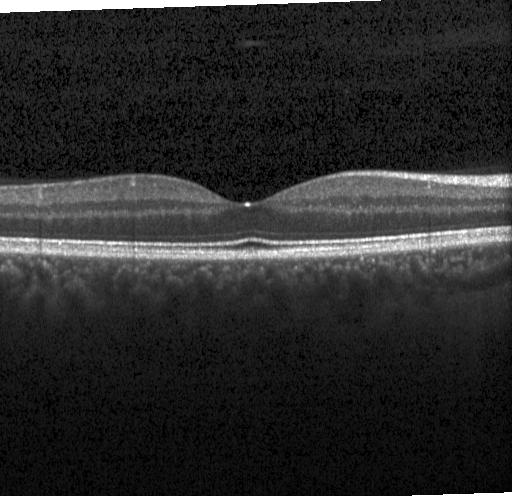
OCT line scan · centered on the fovea — Assessment: neither choroidal neovascularization, diabetic macular edema, nor drusen.